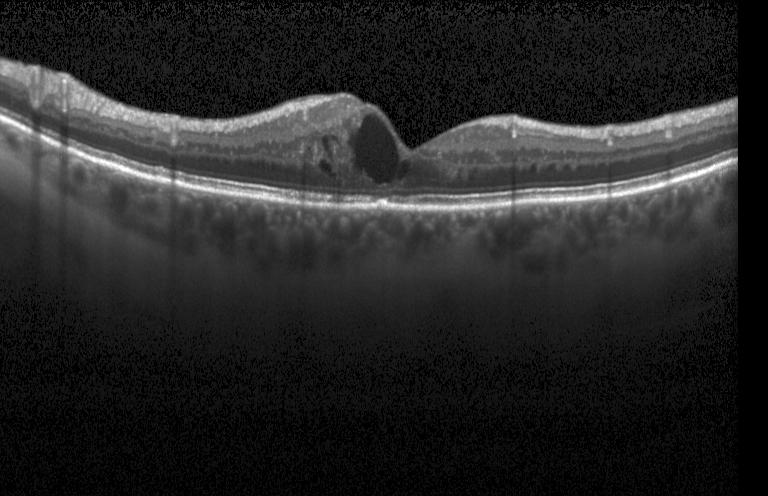
Impression: diabetic macular edema (DME).